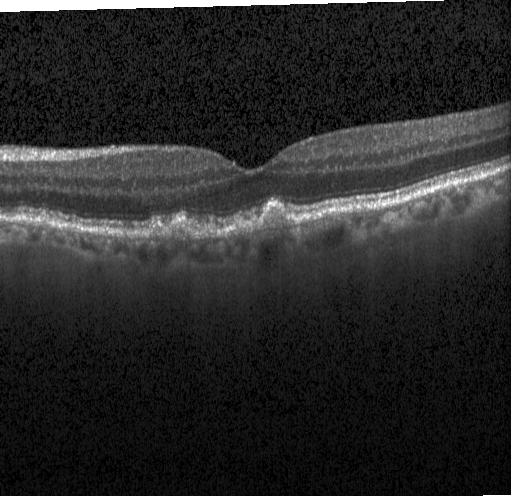
This B-scan demonstrates drusen.